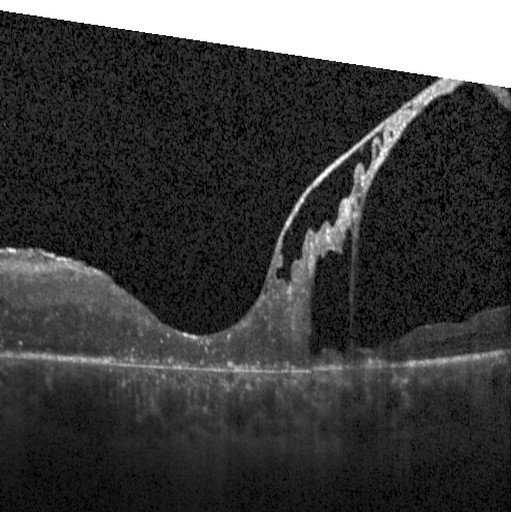

This B-scan demonstrates diabetic macular edema.